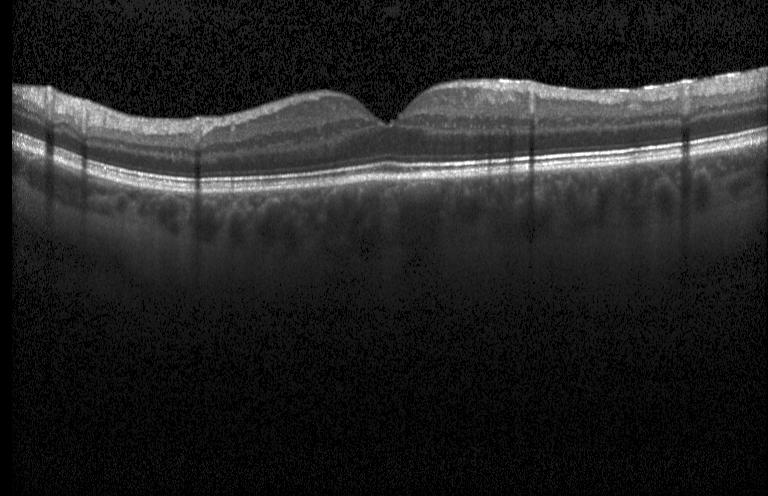

Optical coherence tomography scan · through the macula · Heidelberg Spectralis OCT system · SD-OCT.
Impression: no evidence of choroidal neovascularization, diabetic macular edema, or drusen.